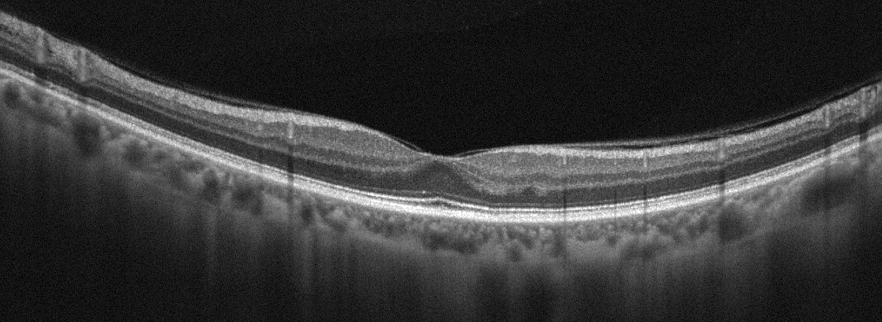
Retinal OCT B-scan · acquired on an Optovue Avanti RTVue XR. This B-scan demonstrates absence of AMD, DME, ERM, RAO, RVO, and vitreomacular interface disease.